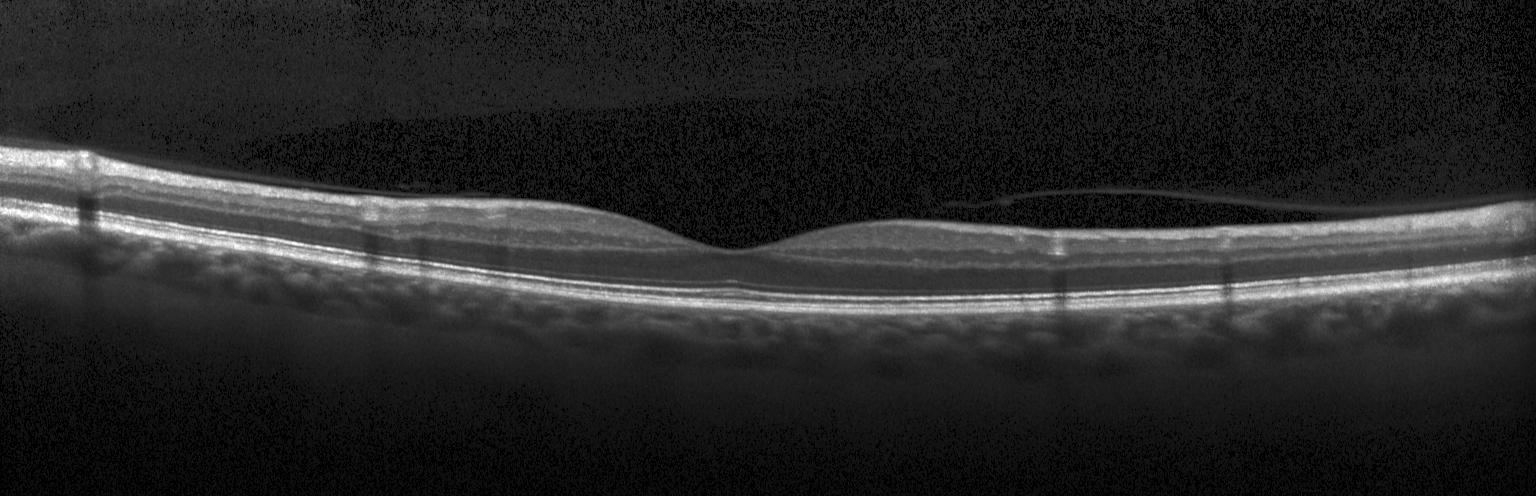

The scan shows no evidence of CNV, DME, or drusen.